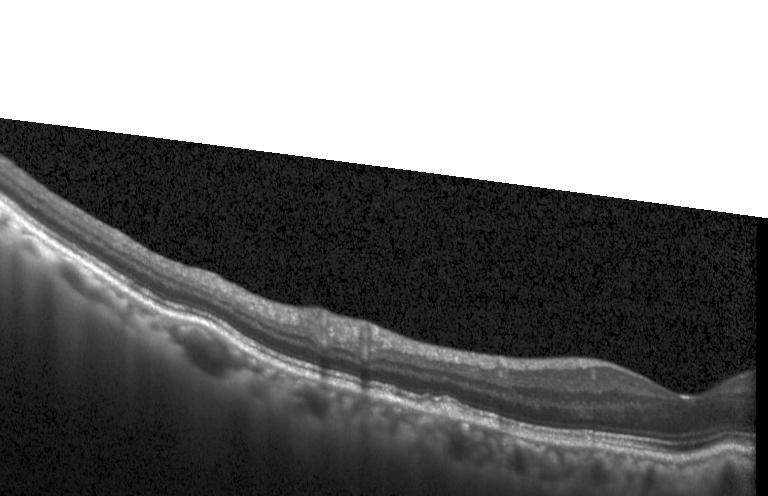 Optical coherence tomography B-scan, SD-OCT.
This B-scan demonstrates sub-RPE drusenoid deposits.